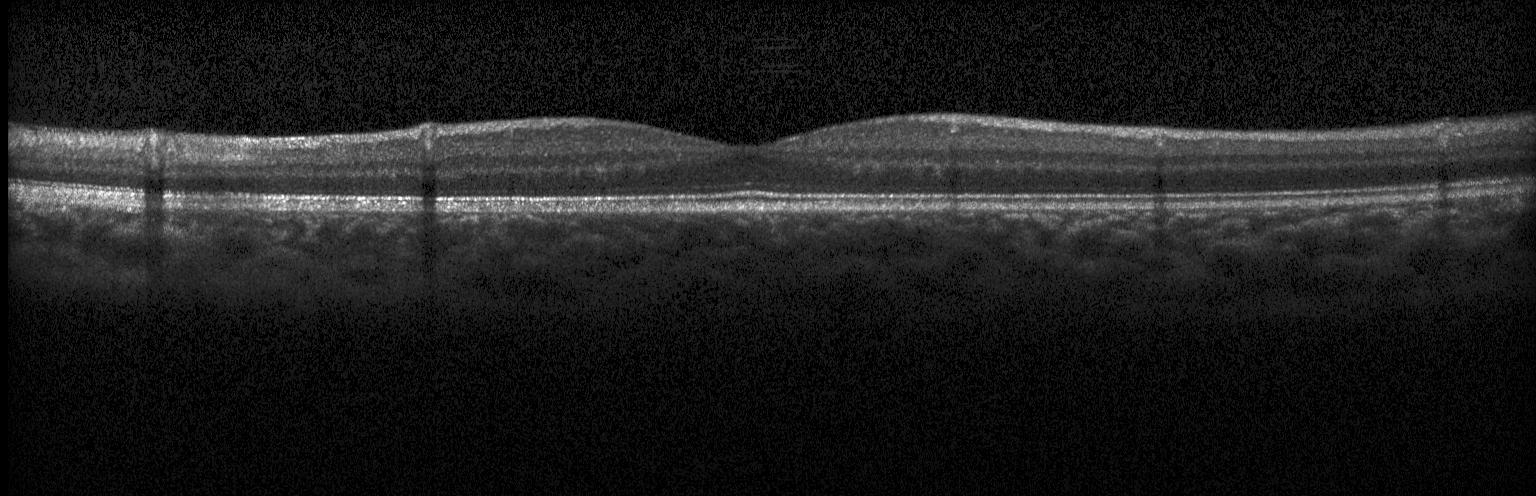
Macular OCT: neither choroidal neovascularization, diabetic macular edema, nor drusen.